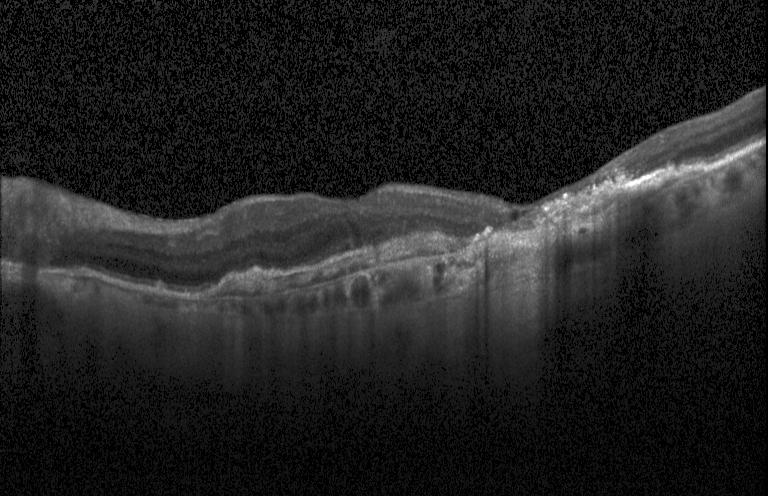

Centered on the fovea; optical coherence tomography B-scan
This B-scan demonstrates a choroidal neovascular membrane.